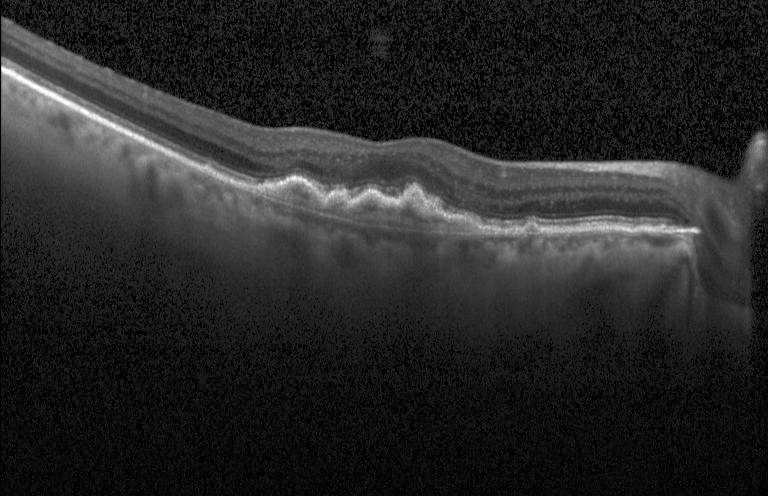

Diagnosis: a choroidal neovascular membrane.